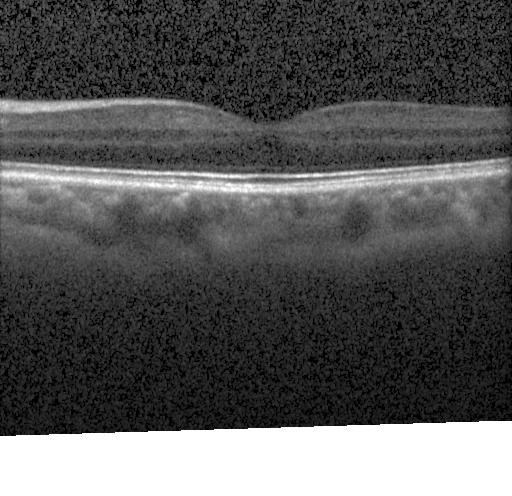 Macular OCT: neither choroidal neovascularization, diabetic macular edema, nor drusen.